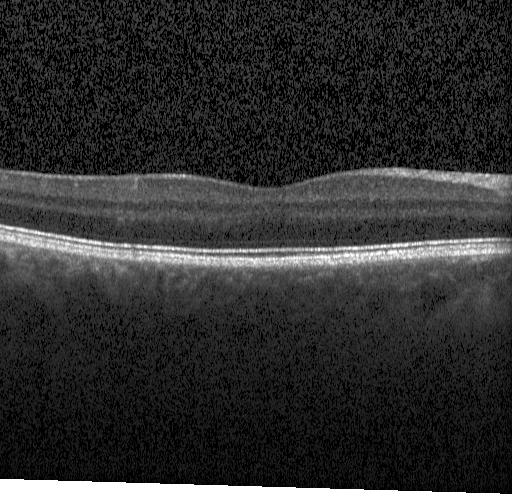 Diagnosis: no choroidal neovascularization, no diabetic macular edema, and no drusen.